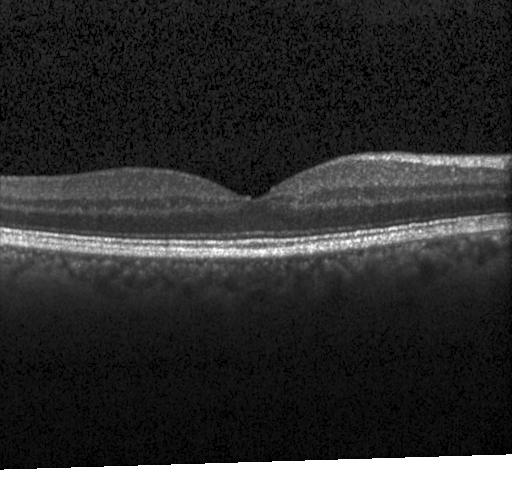 Macular OCT: neither choroidal neovascularization, diabetic macular edema, nor drusen.